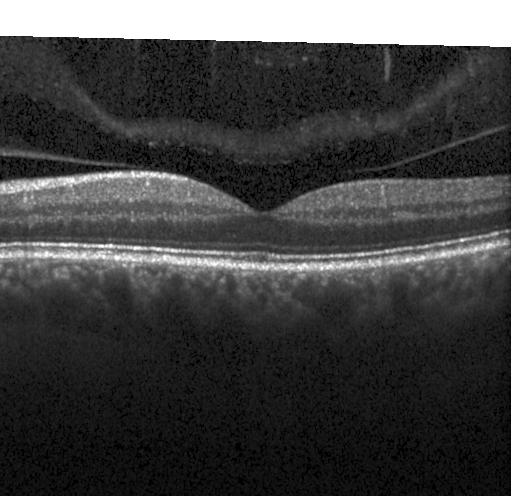
Optical coherence tomography scan · centered on the fovea
OCT finding: no evidence of choroidal neovascularization, diabetic macular edema, or drusen.